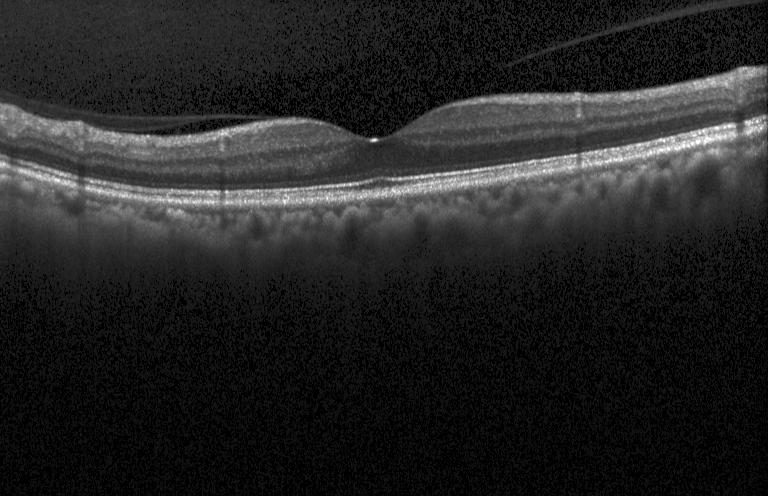
Horizontal scan through the fovea, retinal OCT B-scan, spectral-domain OCT. Impression: no evidence of CNV, DME, or drusen.